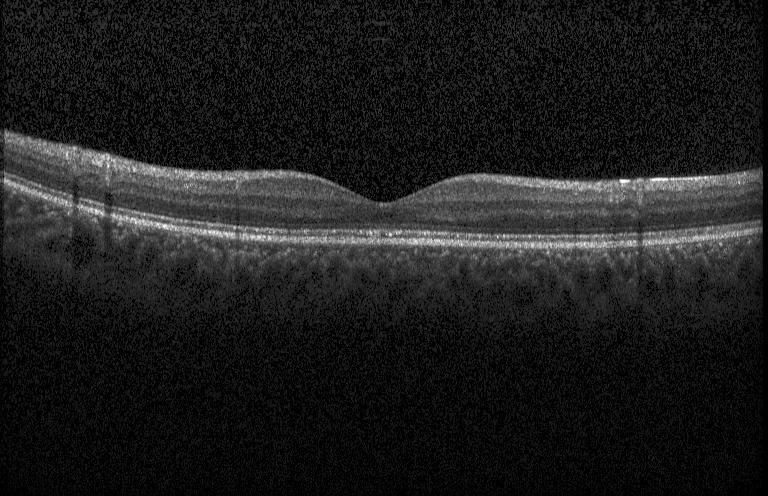
OCT B-scan showing no choroidal neovascularization, diabetic macular edema, or drusen.